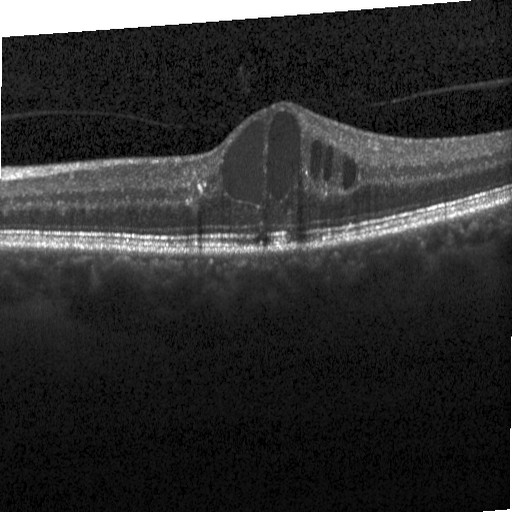 Retinal OCT cross-section
Assessment: diabetic macular edema.